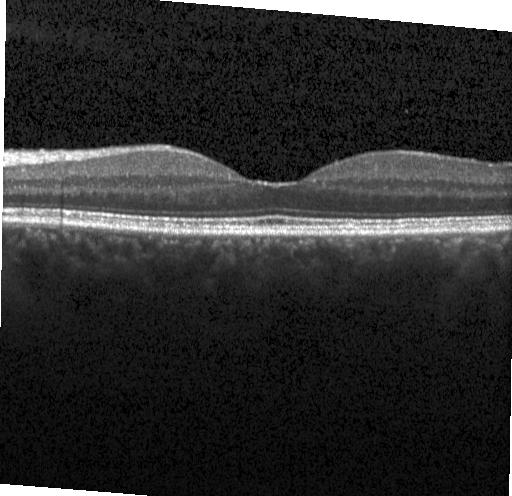 Horizontal scan through the fovea. Optical coherence tomography scan. Spectral-domain optical coherence tomography. Heidelberg Spectralis. Impression: no evidence of CNV, DME, or drusen.